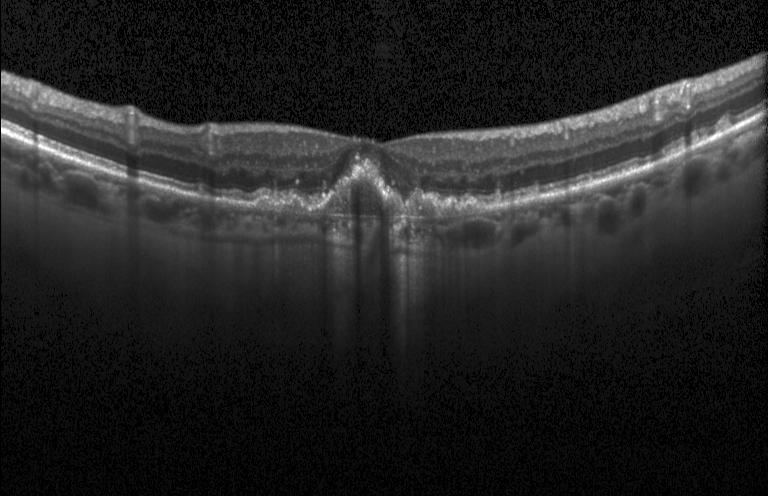
Heidelberg Spectralis. SD-OCT. OCT B-scan. Macular scan — OCT finding: a choroidal neovascular membrane.